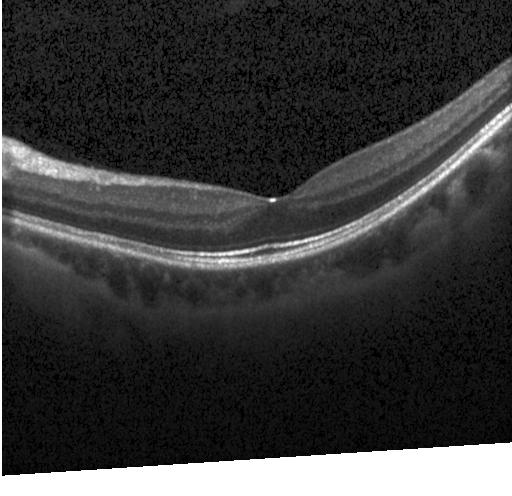

OCT scan showing no CNV, no DME, and no drusen.